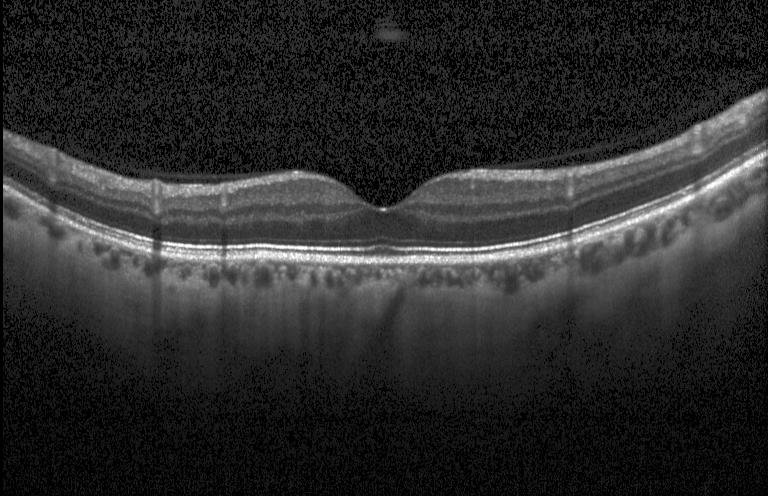

Acquired on a Heidelberg Spectralis; spectral-domain optical coherence tomography; retinal OCT B-scan
The scan shows no choroidal neovascularization, no diabetic macular edema, and no drusen.